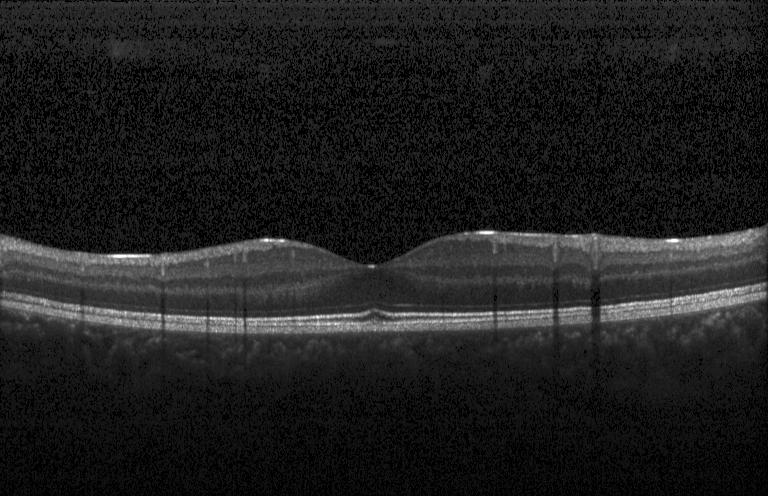
Macular scan, optical coherence tomography scan. The scan shows no choroidal neovascularization, diabetic macular edema, or drusen.